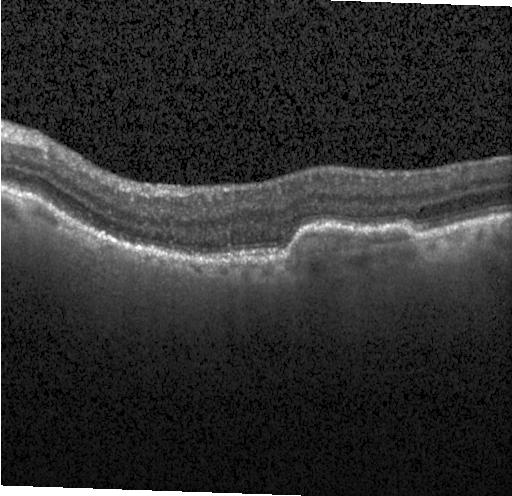 Optical coherence tomography B-scan. Fovea-centered. Heidelberg Spectralis.
Finding: a choroidal neovascular membrane.